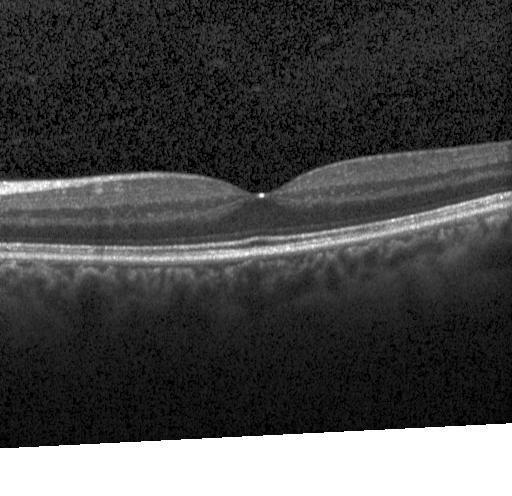 Finding: no evidence of choroidal neovascularization, diabetic macular edema, or drusen.